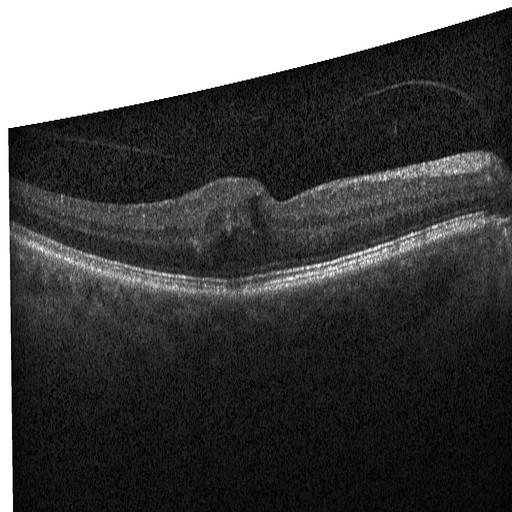 Impression: diabetic macular edema (DME).